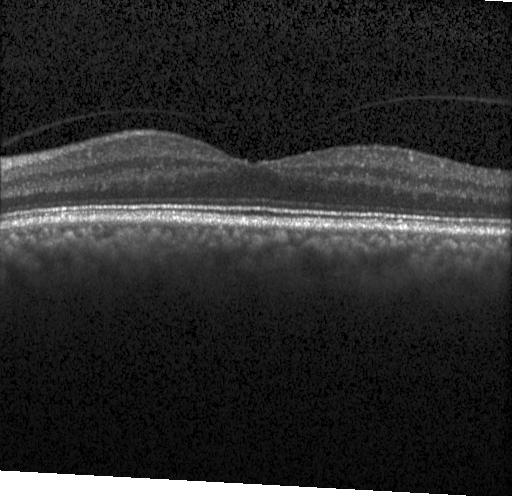

Diagnosis: no choroidal neovascularization, no diabetic macular edema, and no drusen.